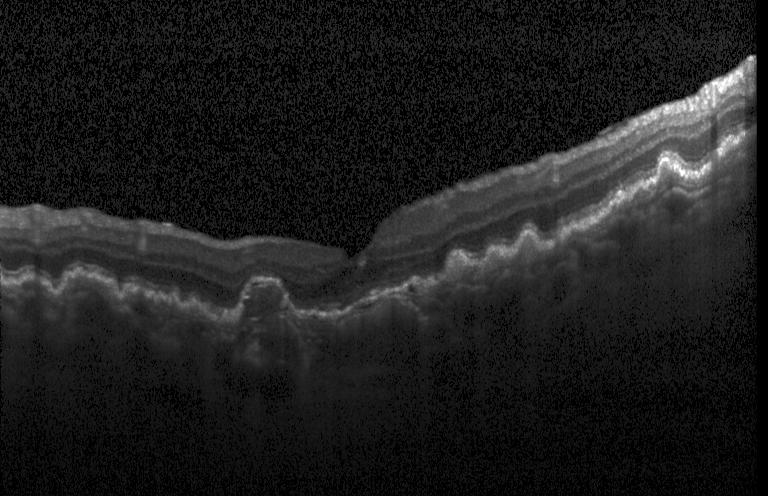

Dx: CNV.